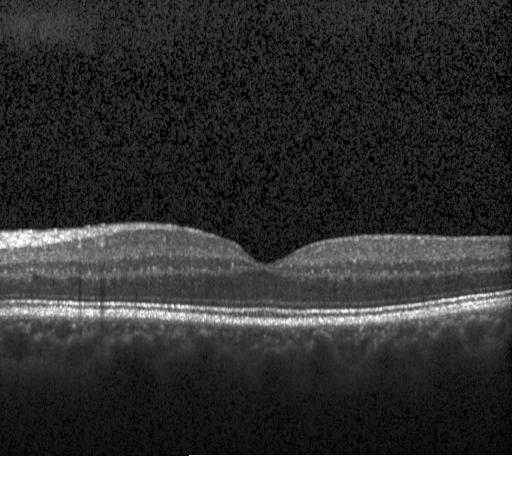

Impression: no choroidal neovascularization, diabetic macular edema, or drusen.